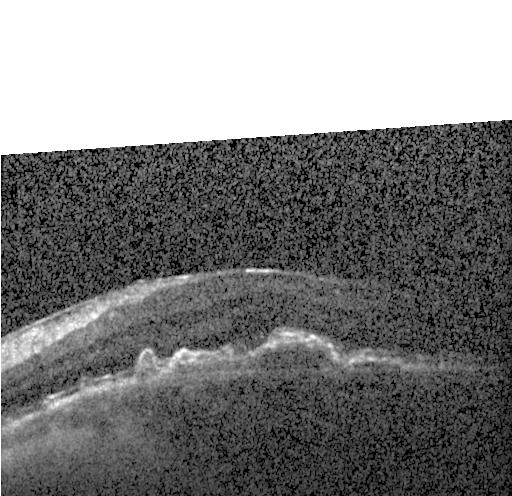
SD-OCT. Optical coherence tomography B-scan — Impression: CNV.